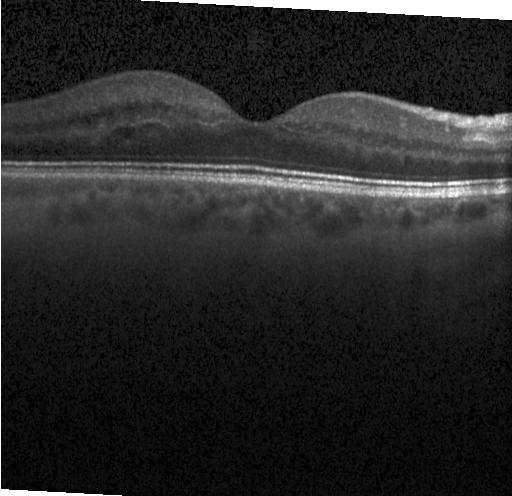

Retinal OCT cross-section — OCT finding: diabetic macular edema (DME).